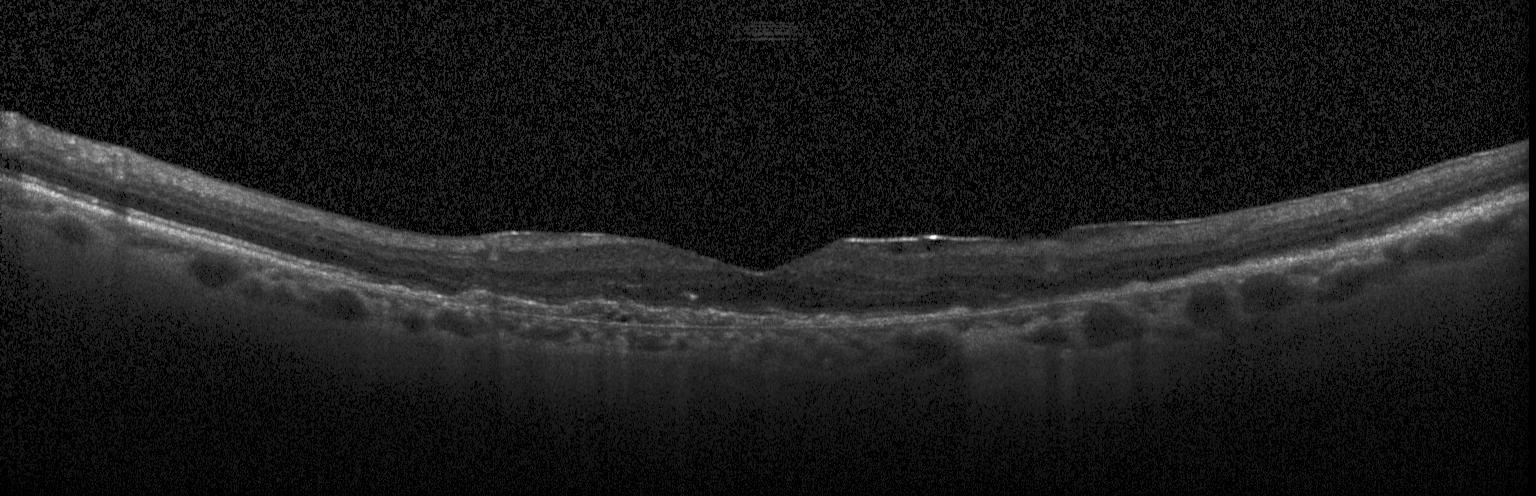 OCT line scan · Heidelberg Spectralis OCT system · SD-OCT
Assessment: choroidal neovascularization.